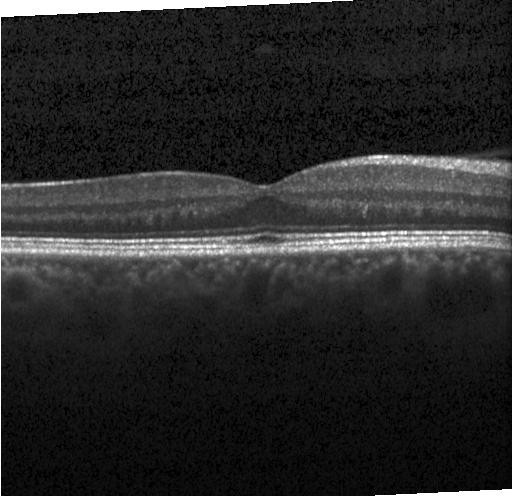 Optical coherence tomography scan
Assessment: no choroidal neovascularization, no diabetic macular edema, and no drusen.